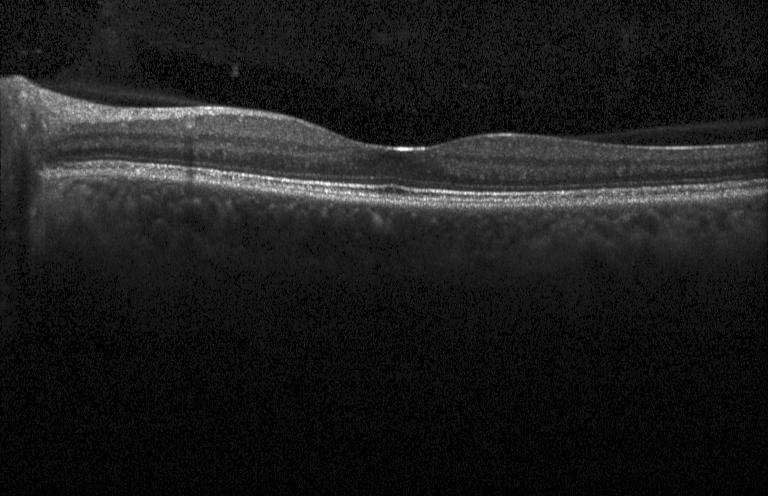

Spectral-domain OCT B-scan: no choroidal neovascularization, diabetic macular edema, or drusen.